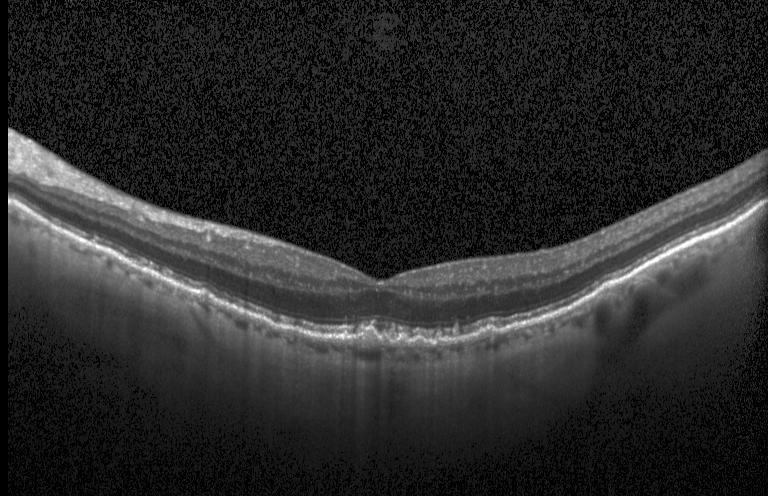
OCT B-scan
Diagnosis: multiple drusen.